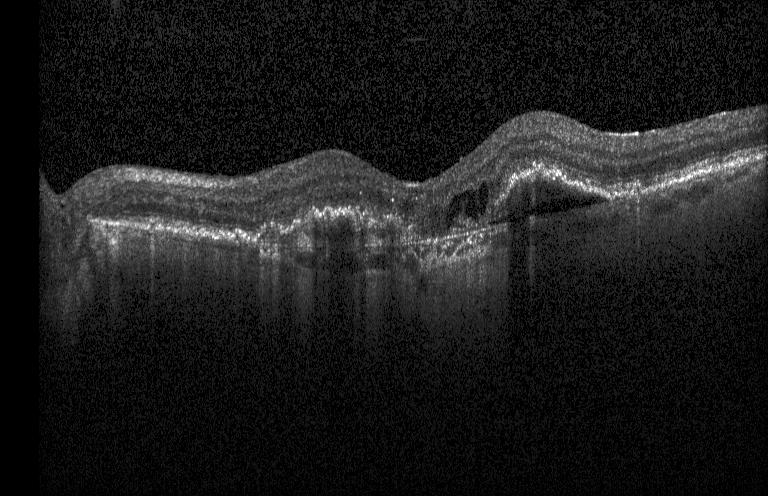 Retinal OCT B-scan; instrument: Heidelberg Spectralis; SD-OCT; macular scan
The scan shows CNV.